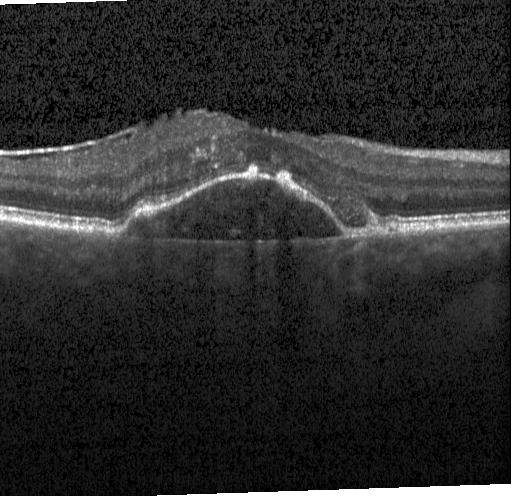 Retinal OCT cross-section showing a choroidal neovascular membrane.